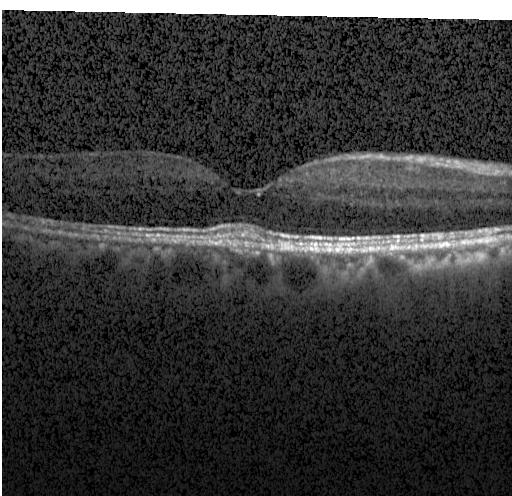
Retinal OCT cross-section
This B-scan demonstrates no choroidal neovascularization, no diabetic macular edema, and no drusen.